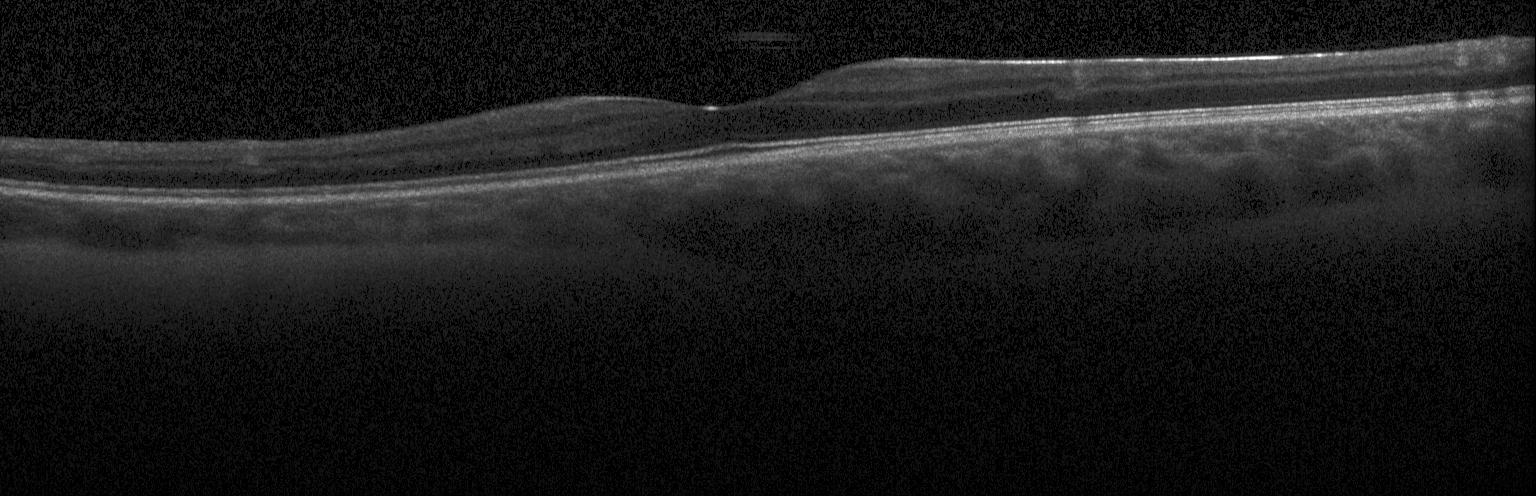
Impression: neither choroidal neovascularization, diabetic macular edema, nor drusen.